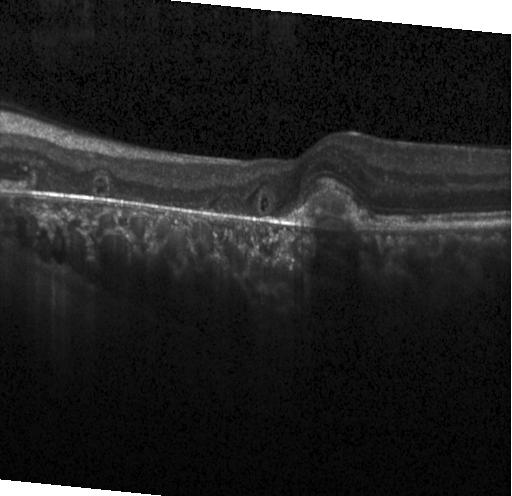 Heidelberg Spectralis. OCT B-scan — Choroidal neovascularization (CNV).